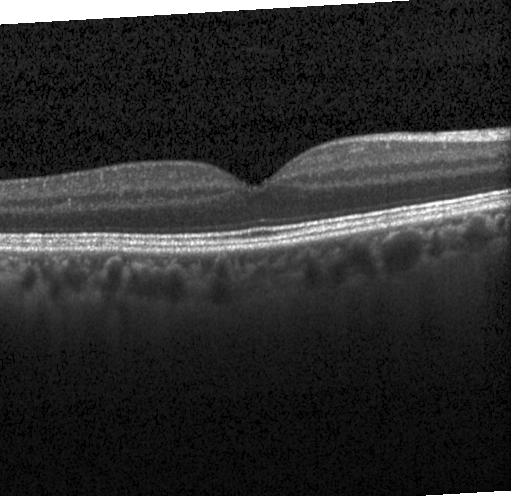 Spectral-domain optical coherence tomography; retinal OCT cross-section; acquired on a Heidelberg Spectralis; fovea-centered.
This B-scan demonstrates no CNV, no DME, and no drusen.